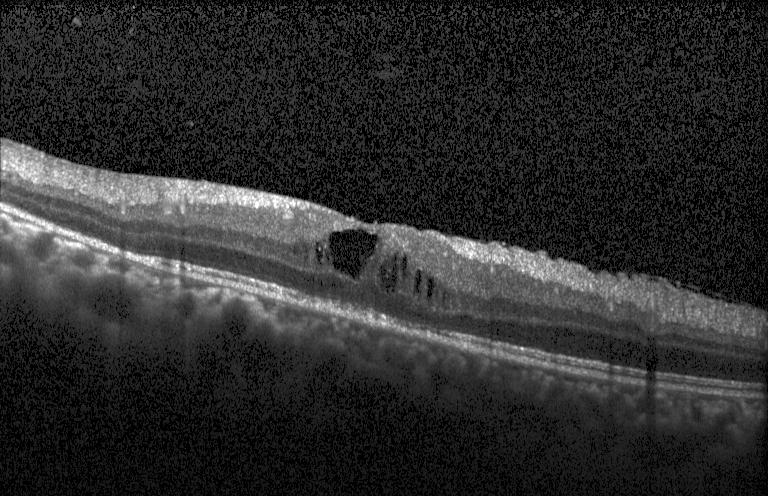
Macular OCT: diabetic macular edema.